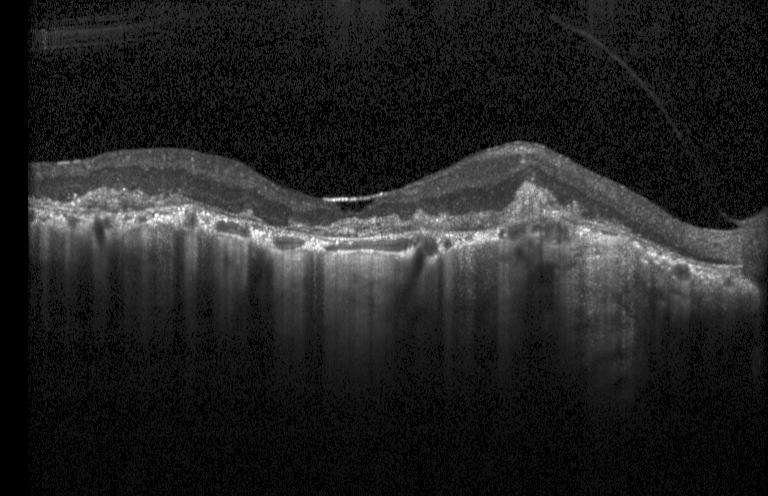
Impression: a choroidal neovascular membrane.